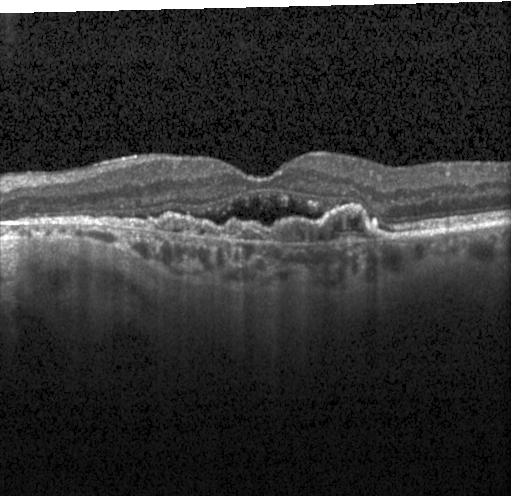 Retinal OCT B-scan; macular scan; spectral-domain optical coherence tomography; instrument: Heidelberg Spectralis
Macular OCT: CNV.